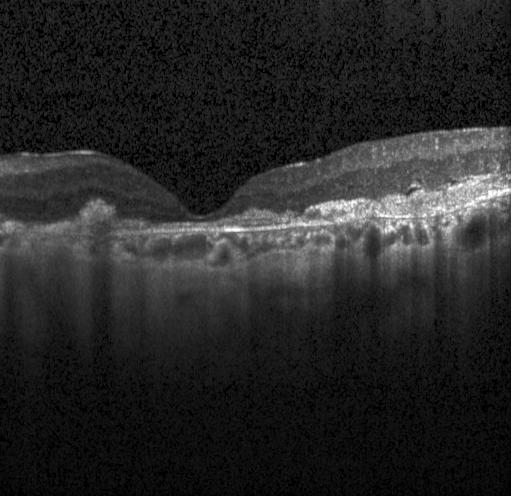

Acquired on a Heidelberg Spectralis · spectral-domain OCT · OCT B-scan · fovea-centered — Assessment: a choroidal neovascular membrane.